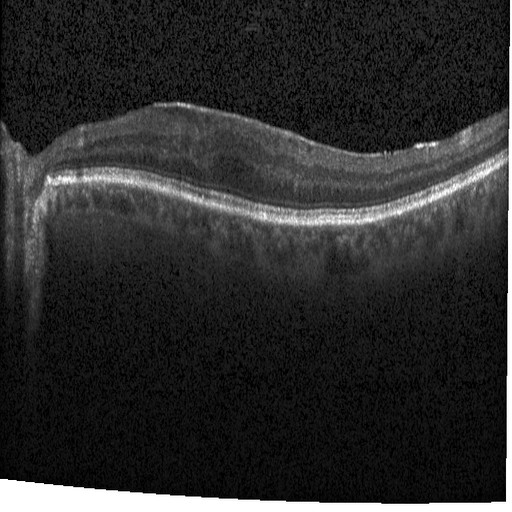 Assessment: DME.